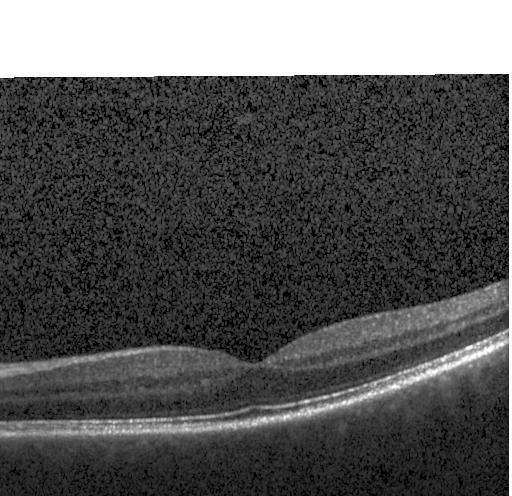

Spectral-domain OCT B-scan: no choroidal neovascularization, no diabetic macular edema, and no drusen.